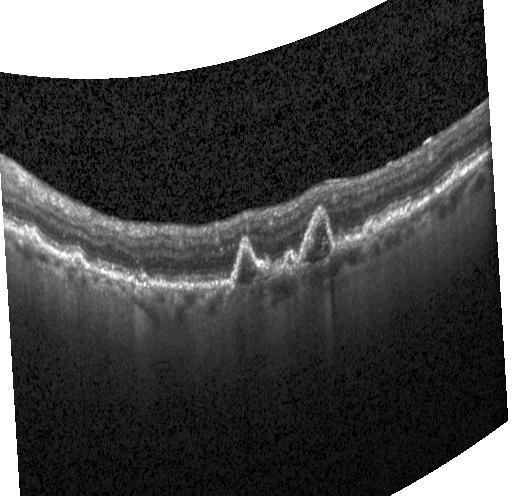

Through the macula. Spectral-domain optical coherence tomography. Optical coherence tomography B-scan. Instrument: Heidelberg Spectralis.
Dx: choroidal neovascularization (CNV).